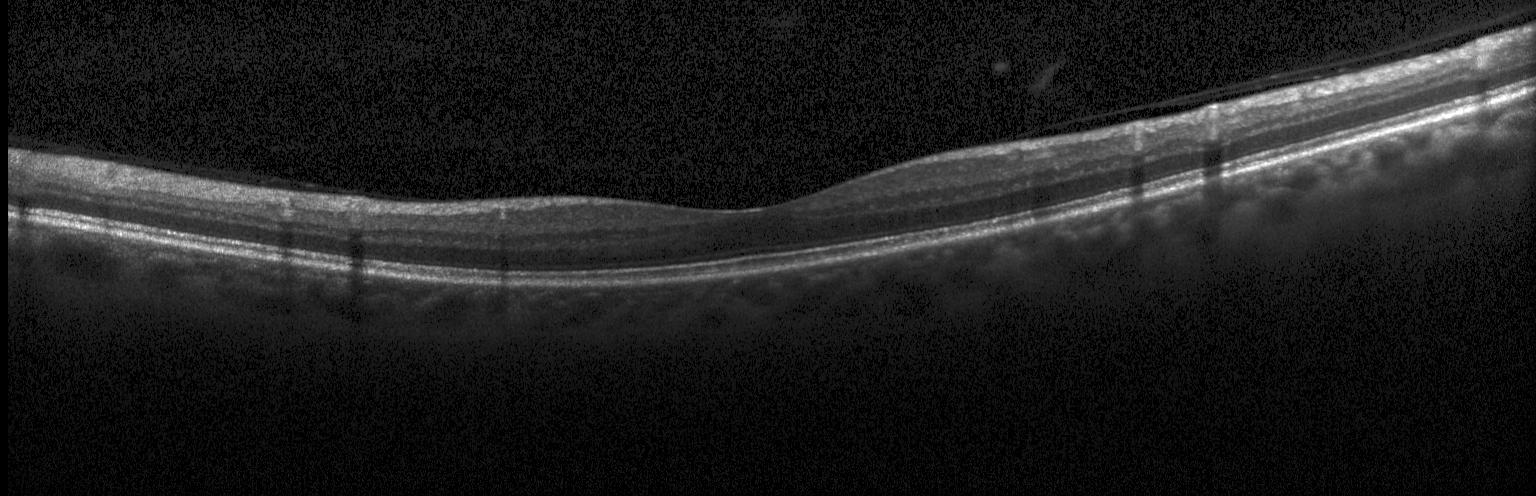

Assessment: no CNV, no DME, and no drusen.